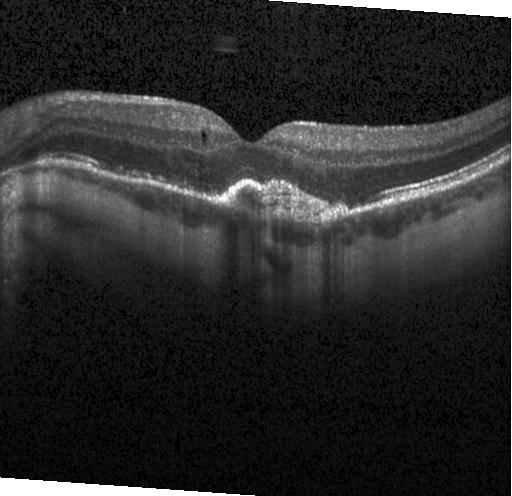

Impression: CNV.